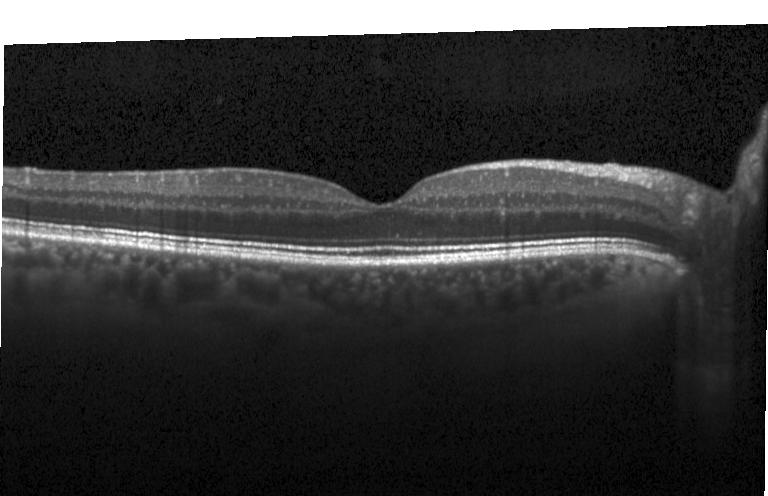

Macular OCT demonstrating no choroidal neovascularization, diabetic macular edema, or drusen.